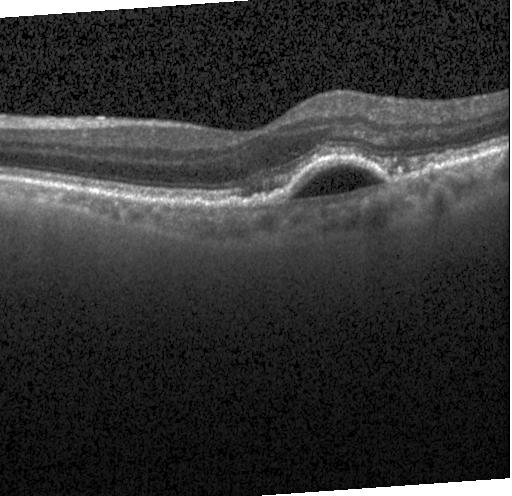
Horizontal scan through the fovea, spectral-domain OCT, retinal OCT B-scan.
Finding: choroidal neovascularization (CNV).